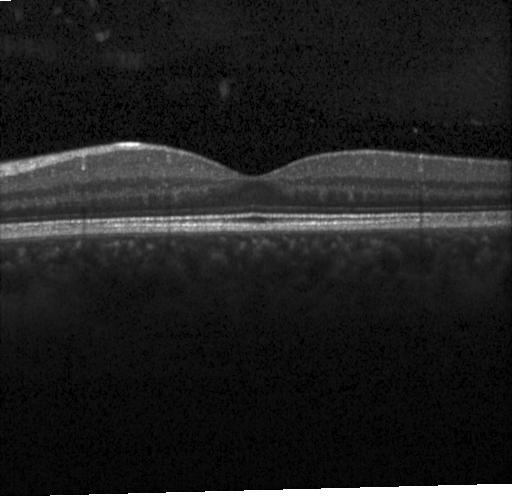
OCT line scan
No evidence of CNV, DME, or drusen.